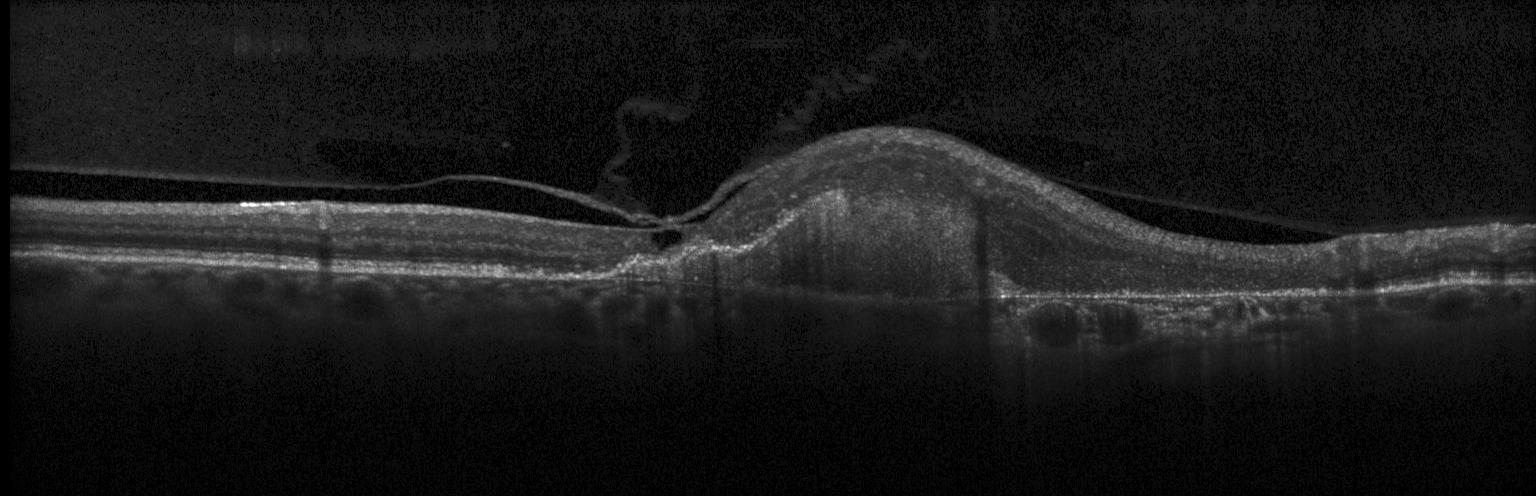 Optical coherence tomography scan, spectral-domain OCT — Diagnosis: a choroidal neovascular membrane.